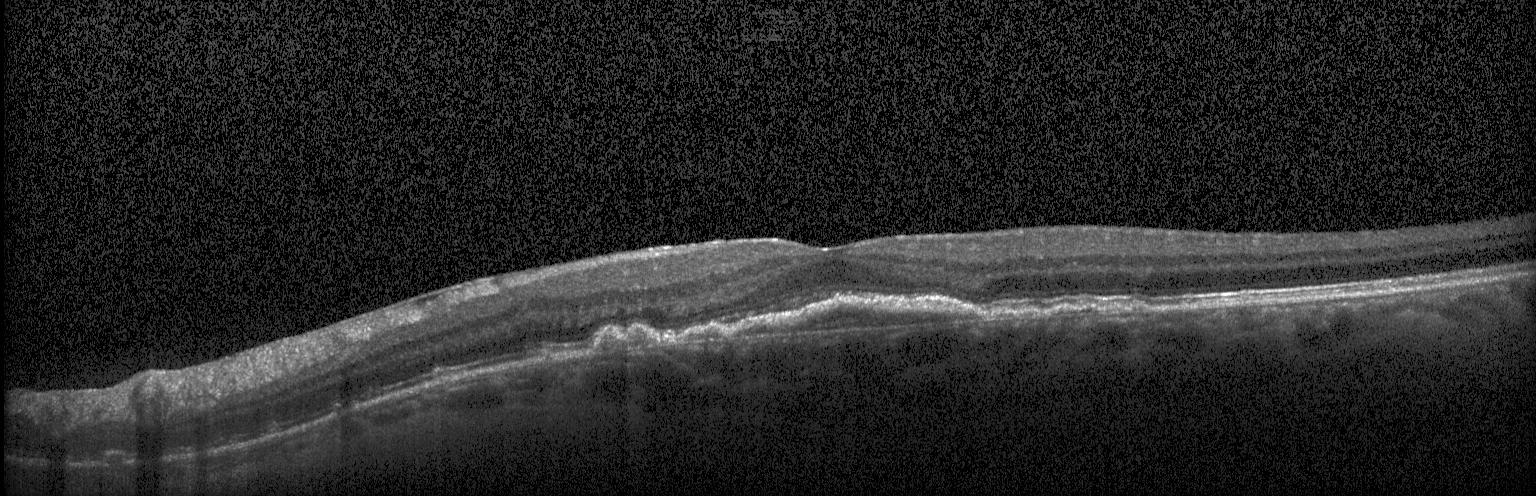 OCT line scan
Dx: CNV.